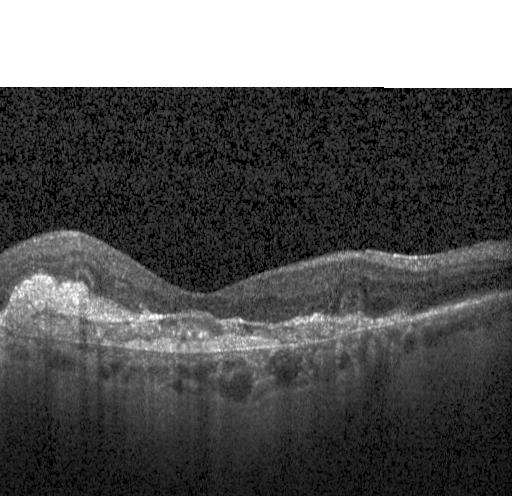
OCT B-scan showing CNV.